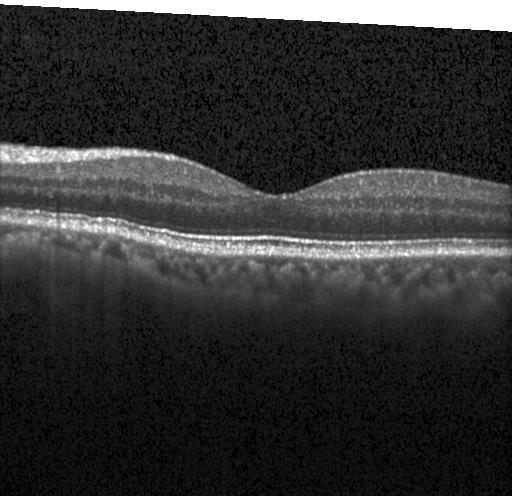 Fovea-centered · acquired on a Heidelberg Spectralis · OCT B-scan.
Dx: no evidence of CNV, DME, or drusen.